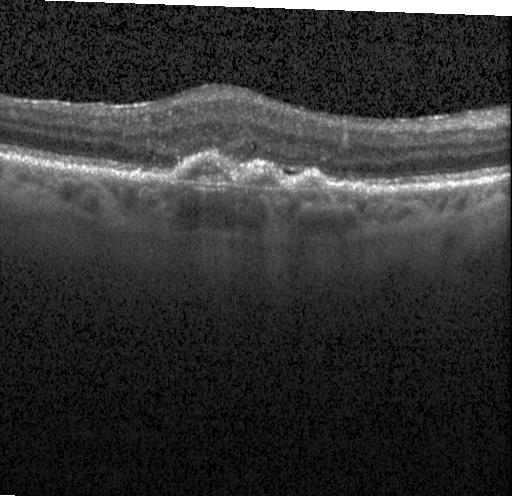
Horizontal scan through the fovea · instrument: Heidelberg Spectralis · SD-OCT · optical coherence tomography B-scan.
Diagnosis: a choroidal neovascular membrane.